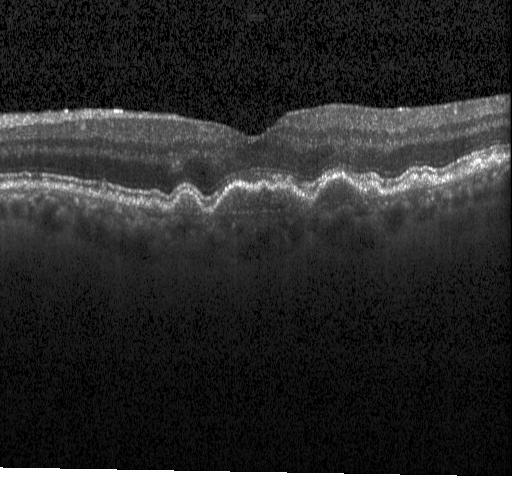 Retinal OCT cross-section. This B-scan demonstrates sub-RPE drusenoid deposits.